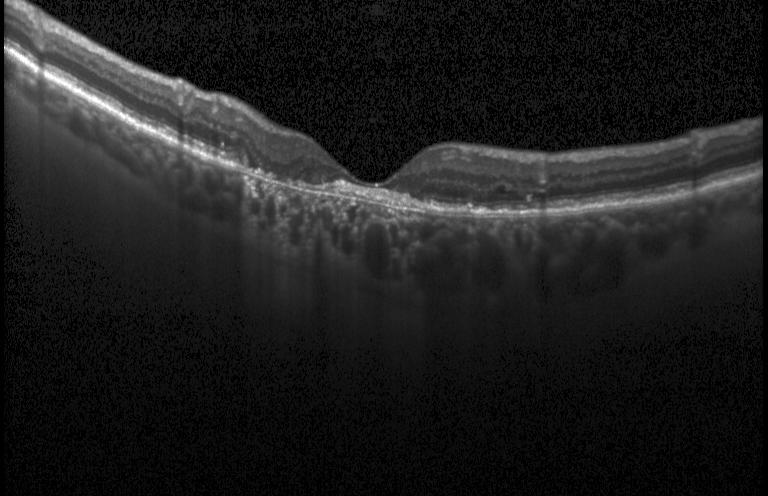
OCT line scan
The scan shows CNV.